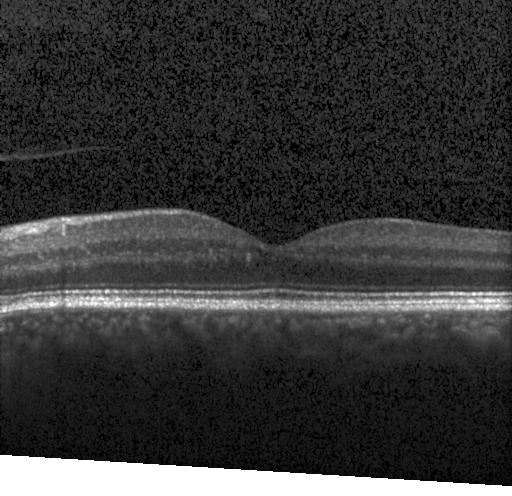 OCT finding: no choroidal neovascularization, no diabetic macular edema, and no drusen.